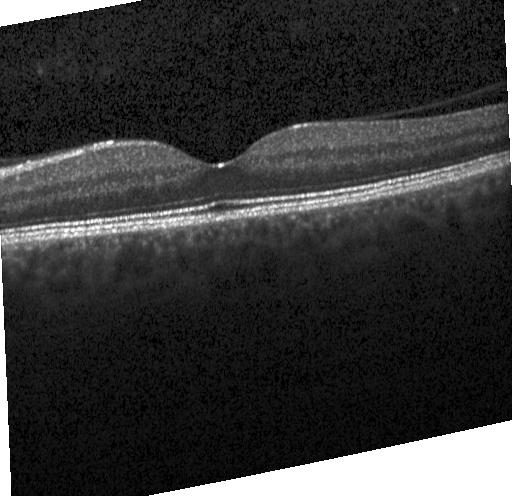

Macular scan; spectral-domain OCT; retinal OCT cross-section; Heidelberg Spectralis OCT system. Diagnosis: no choroidal neovascularization, diabetic macular edema, or drusen.